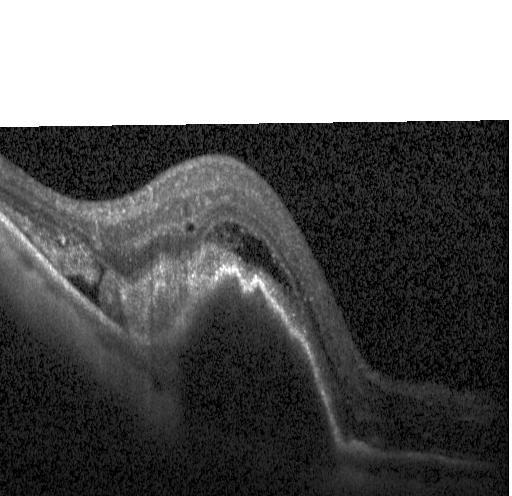

Retinal OCT B-scan, centered on the fovea, spectral-domain optical coherence tomography, Heidelberg Spectralis OCT system
A choroidal neovascular membrane.